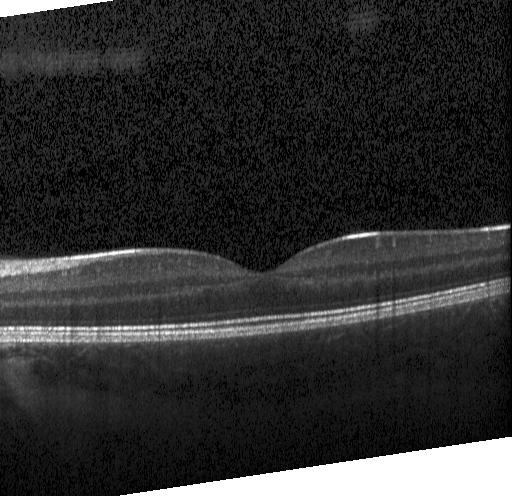

OCT line scan
Finding: no CNV, DME, or drusen.